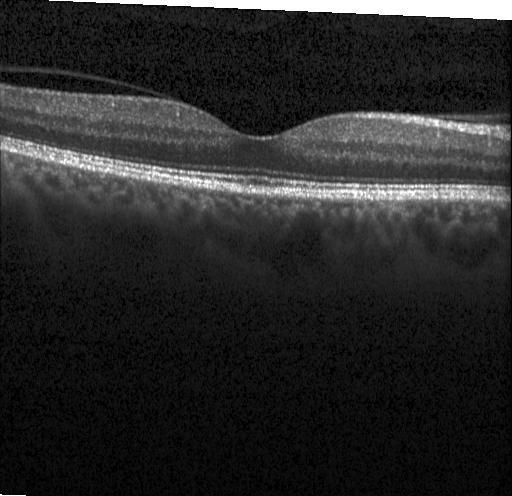
Horizontal scan through the fovea; retinal OCT cross-section; spectral-domain optical coherence tomography
This B-scan demonstrates neither CNV, DME, nor drusen.